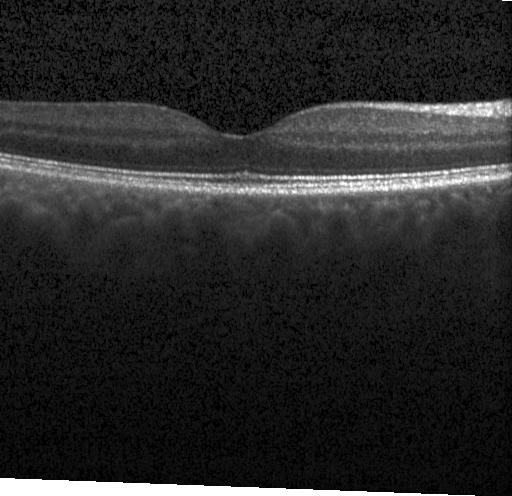

Heidelberg Spectralis · spectral-domain optical coherence tomography · OCT line scan · macular scan
Diagnosis: no evidence of choroidal neovascularization, diabetic macular edema, or drusen.